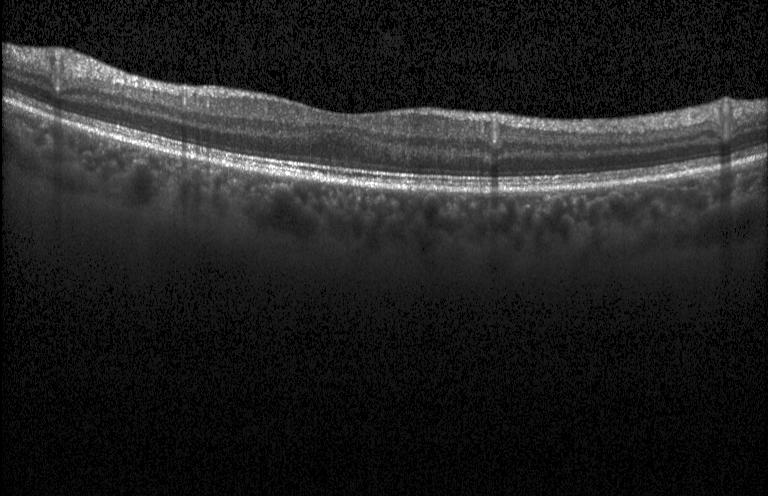 OCT line scan
The scan shows no choroidal neovascularization, diabetic macular edema, or drusen.